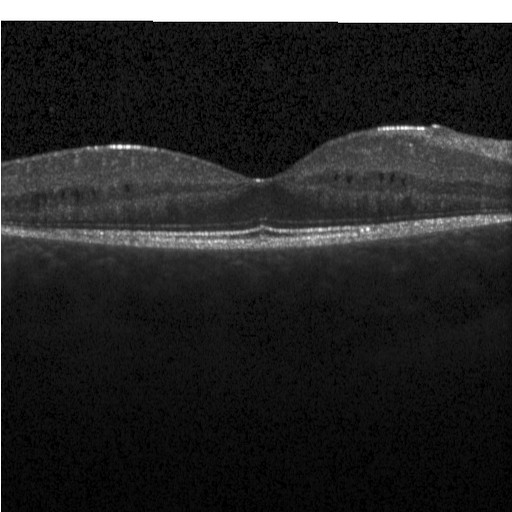

Spectral-domain OCT; optical coherence tomography scan.
Impression: diabetic macular edema.